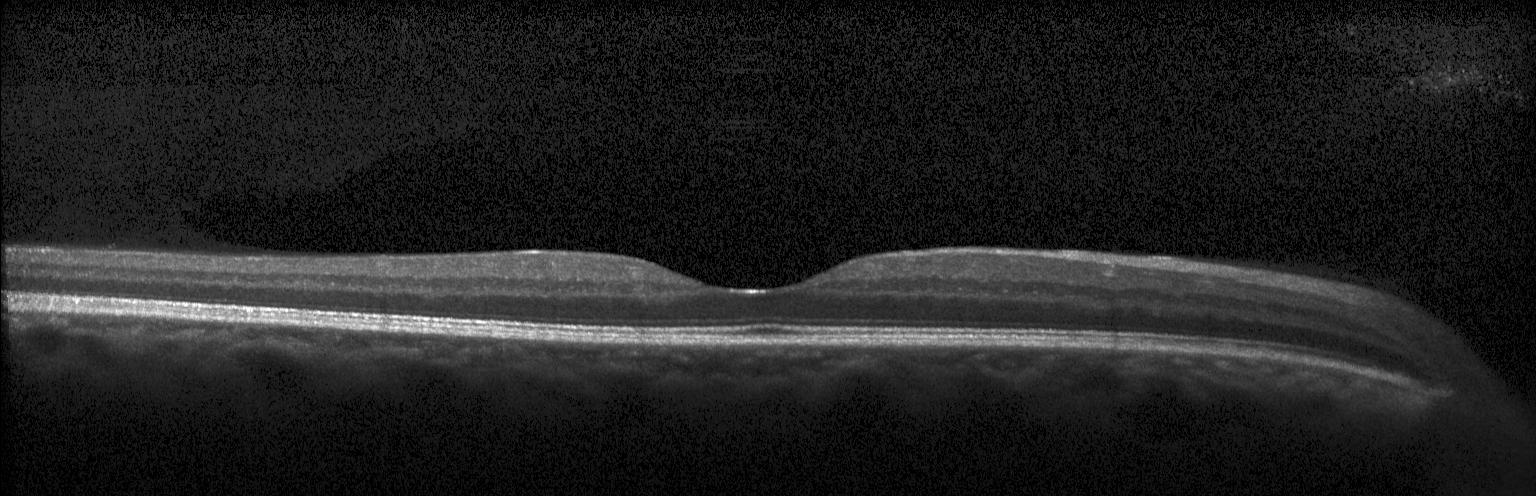 Diagnosis: no choroidal neovascularization, no diabetic macular edema, and no drusen.